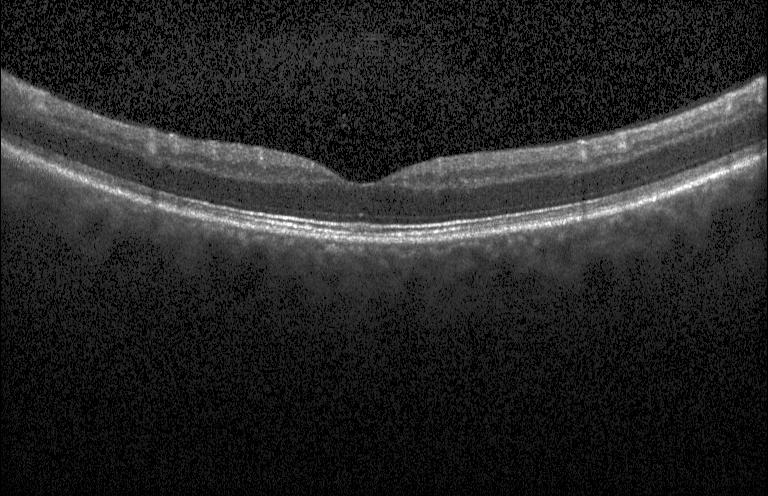

OCT B-scan · macular scan · spectral-domain OCT.
The scan shows no evidence of choroidal neovascularization, diabetic macular edema, or drusen.